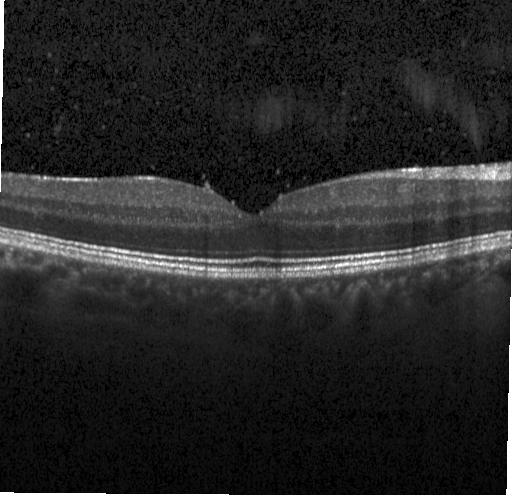

Finding: neither CNV, DME, nor drusen.